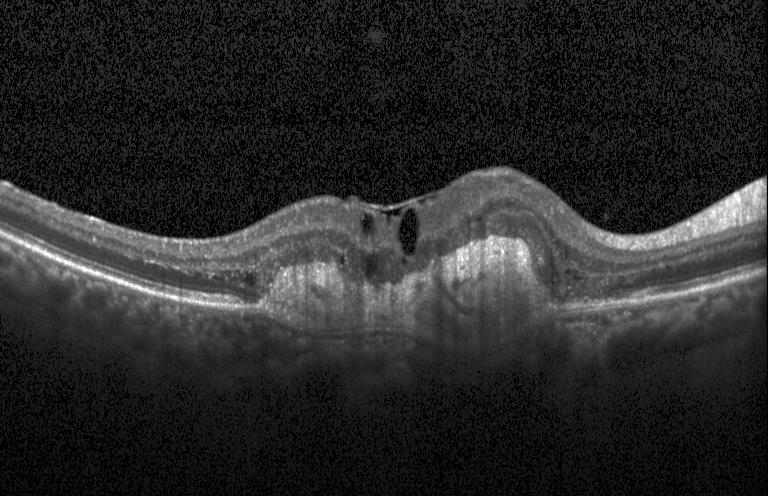

OCT B-scan.
This B-scan demonstrates a choroidal neovascular membrane.